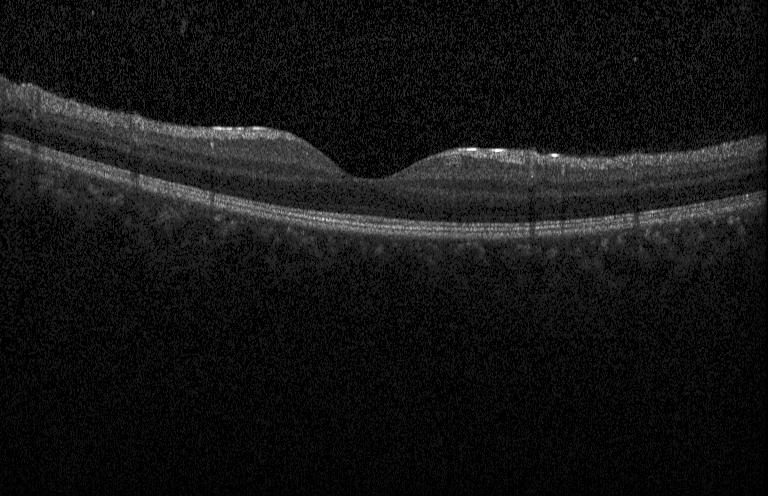

This B-scan demonstrates neither choroidal neovascularization, diabetic macular edema, nor drusen.